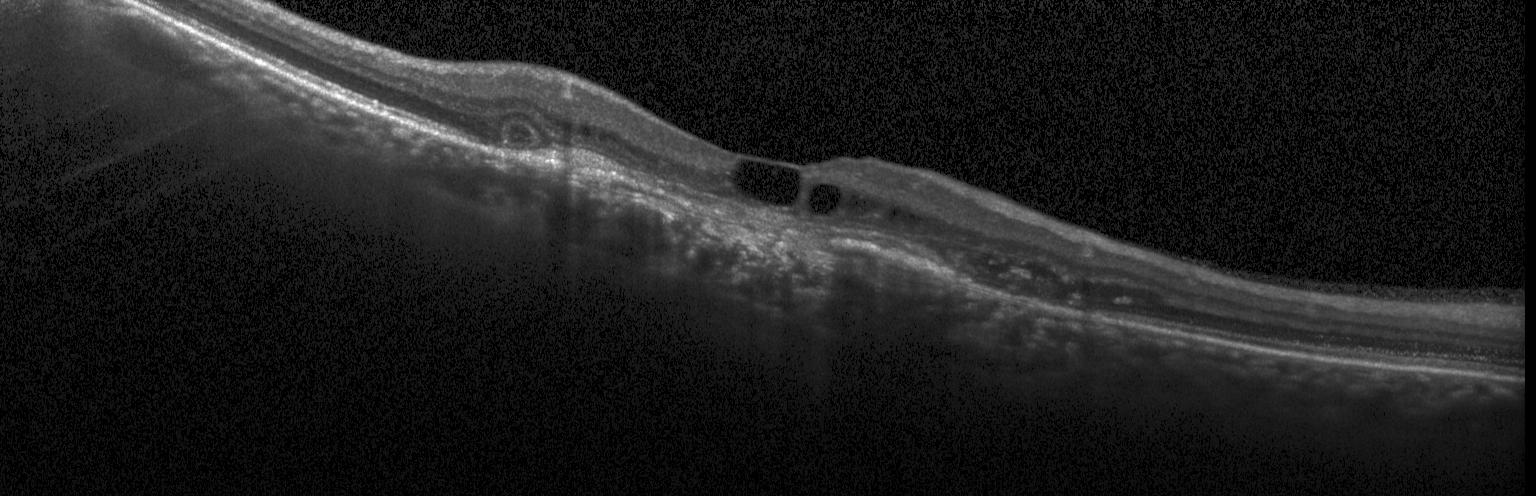 Diagnosis: choroidal neovascularization (CNV).